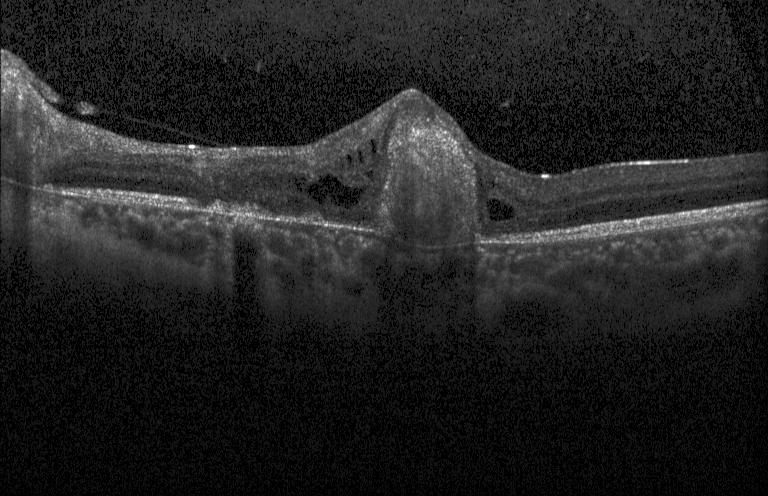
Finding: choroidal neovascularization (CNV).